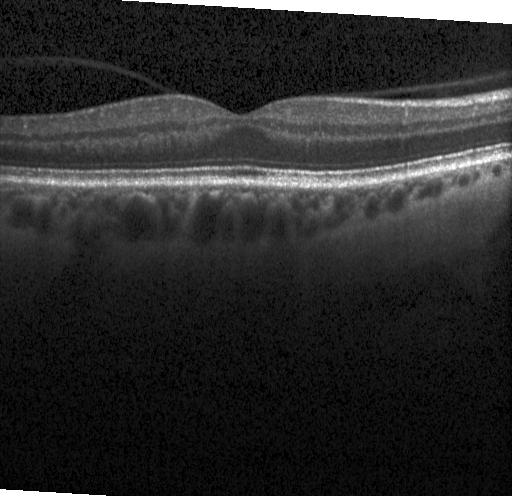

Diagnosis: no choroidal neovascularization, no diabetic macular edema, and no drusen.